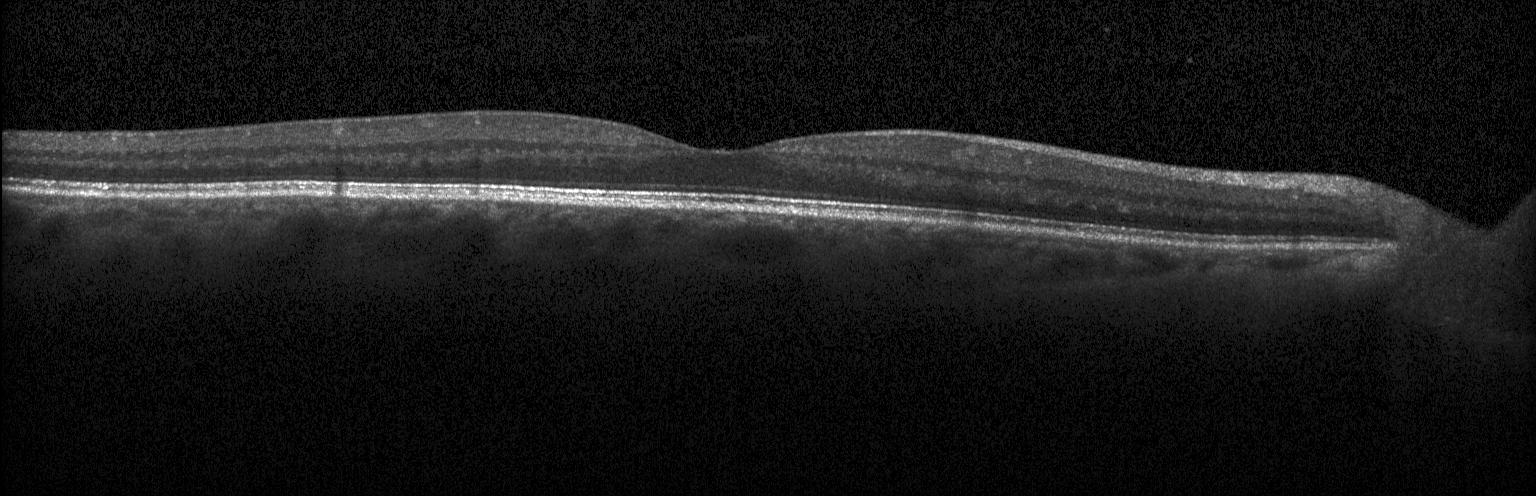

Spectral-domain optical coherence tomography, macular scan, acquired on a Heidelberg Spectralis, optical coherence tomography scan.
Impression: neither choroidal neovascularization, diabetic macular edema, nor drusen.